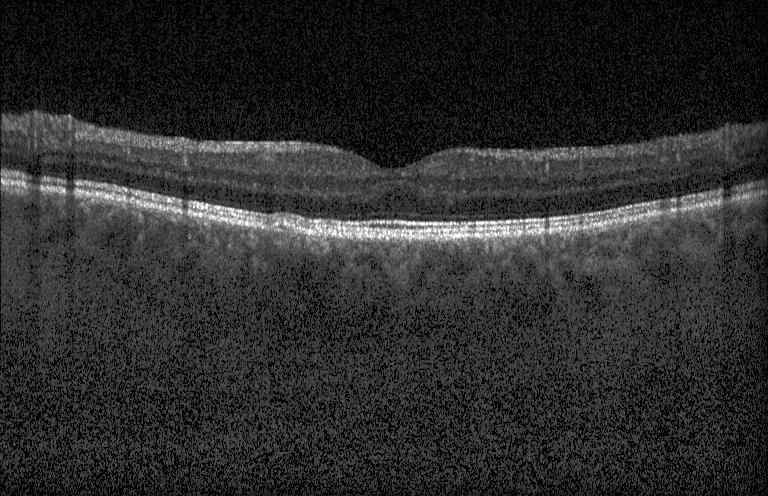
Optical coherence tomography B-scan, horizontal scan through the fovea, spectral-domain optical coherence tomography, instrument: Heidelberg Spectralis — Macular OCT: no evidence of CNV, DME, or drusen.